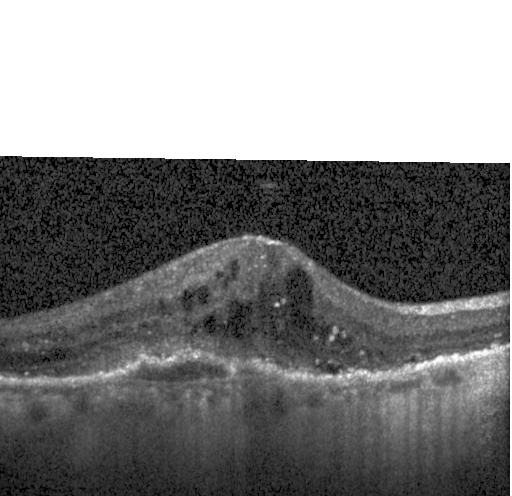 OCT B-scan
OCT finding: a choroidal neovascular membrane.